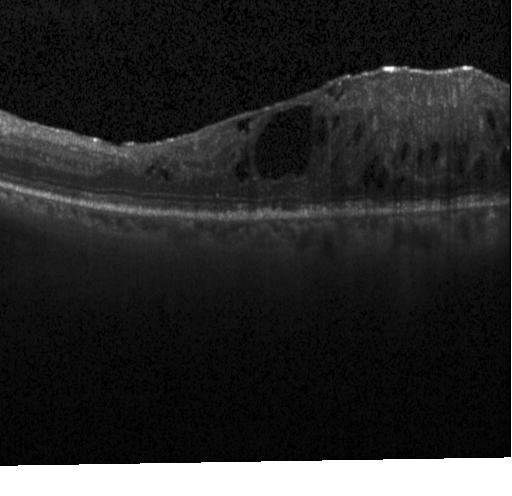 Acquired on a Heidelberg Spectralis · OCT B-scan. Impression: diabetic macular edema.